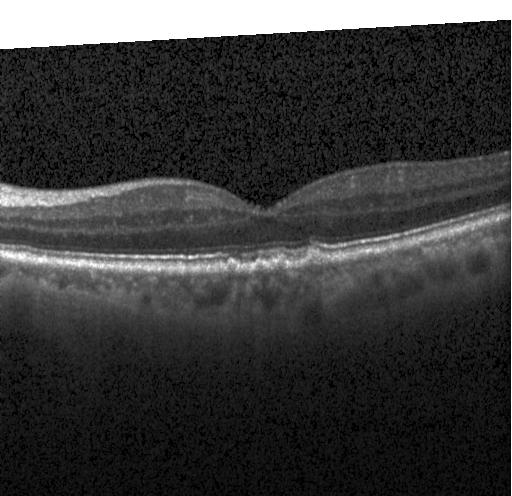

Centered on the fovea, spectral-domain optical coherence tomography, OCT line scan — Sub-RPE drusenoid deposits.